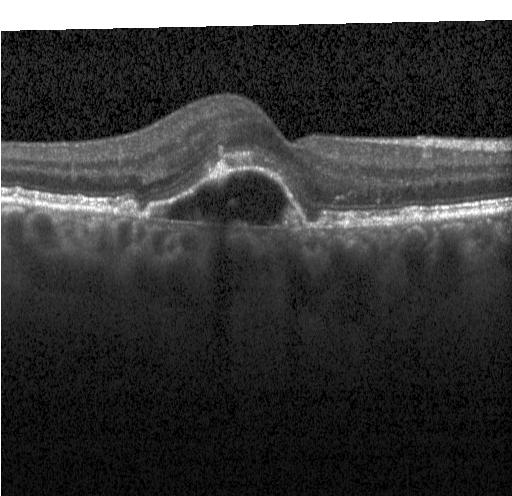

SD-OCT. OCT line scan. Heidelberg Spectralis. Finding: a choroidal neovascular membrane.